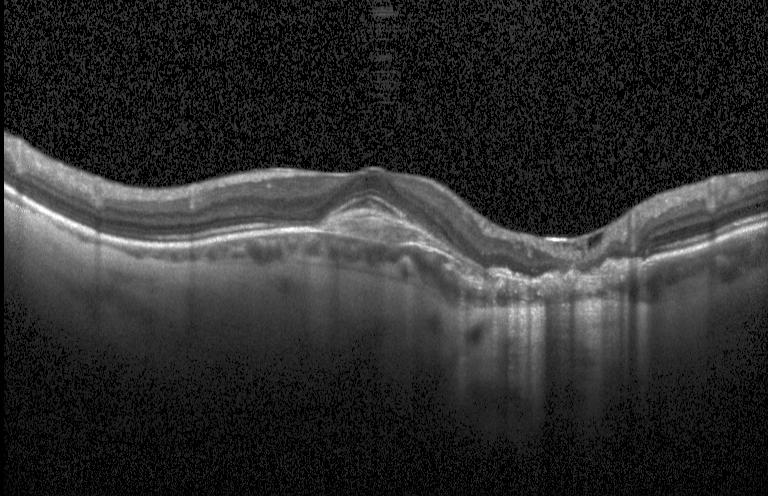
Macular scan · retinal OCT cross-section · acquired on a Heidelberg Spectralis · spectral-domain OCT
Finding: a choroidal neovascular membrane.